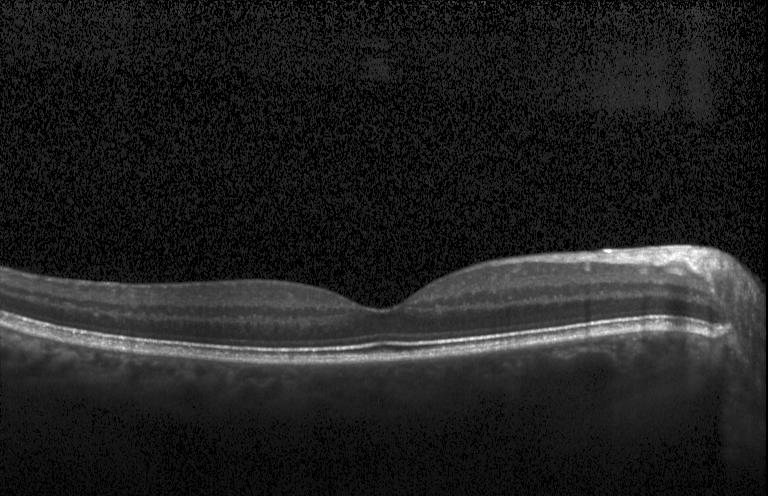 Finding: no CNV, no DME, and no drusen.